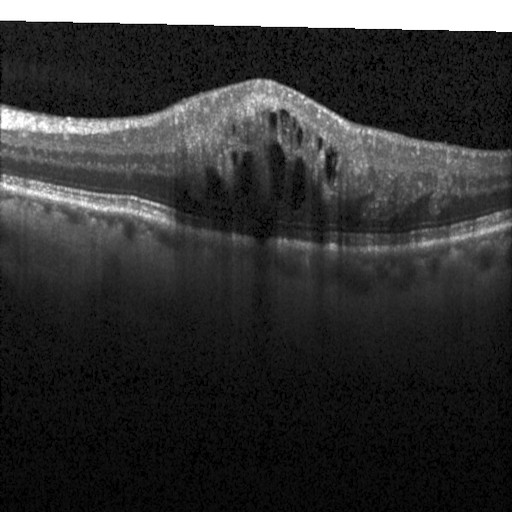 Macular OCT demonstrating diabetic macular edema (DME).